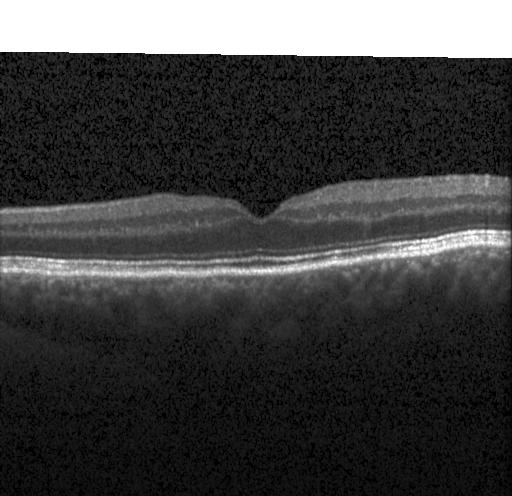 Impression: no evidence of choroidal neovascularization, diabetic macular edema, or drusen.